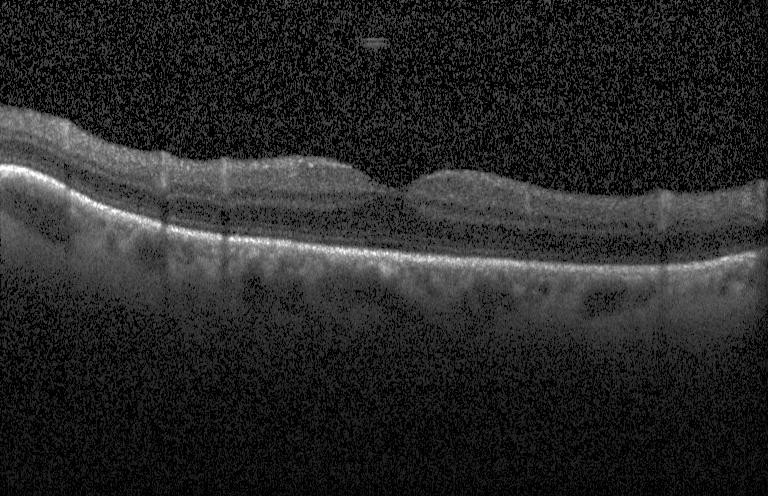 Macular OCT demonstrating neither choroidal neovascularization, diabetic macular edema, nor drusen.